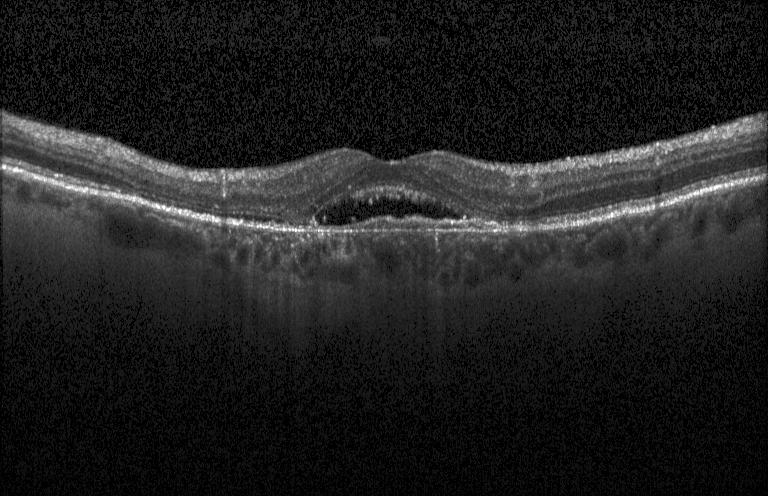 Macular scan; acquired on a Heidelberg Spectralis; retinal OCT cross-section.
Macular OCT: a choroidal neovascular membrane.